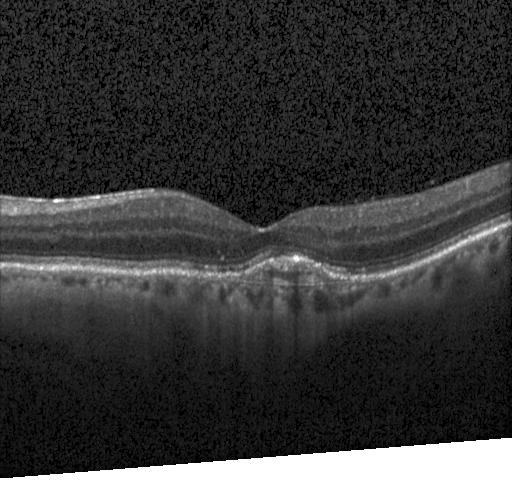 Finding: choroidal neovascularization.